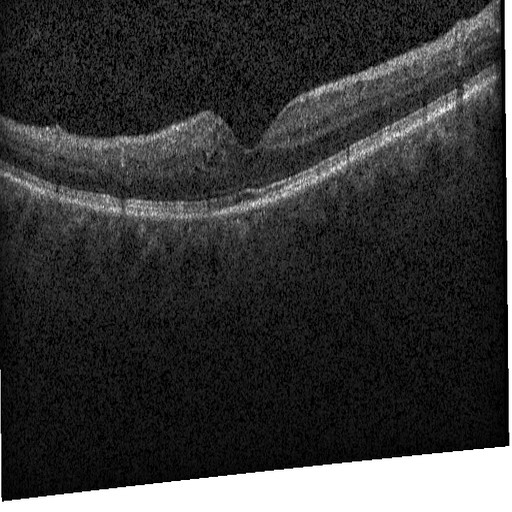
Impression: diabetic macular edema.